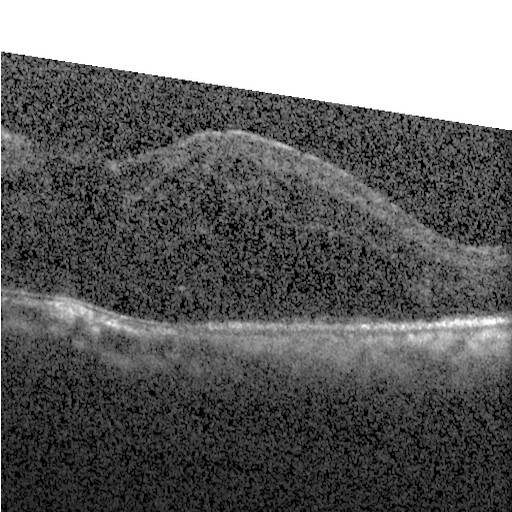
Optical coherence tomography B-scan. OCT finding: DME.